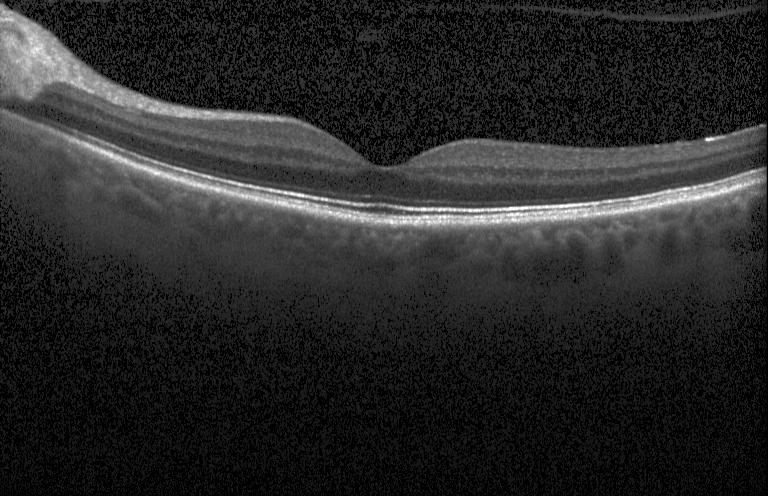
OCT B-scan showing no choroidal neovascularization, diabetic macular edema, or drusen.